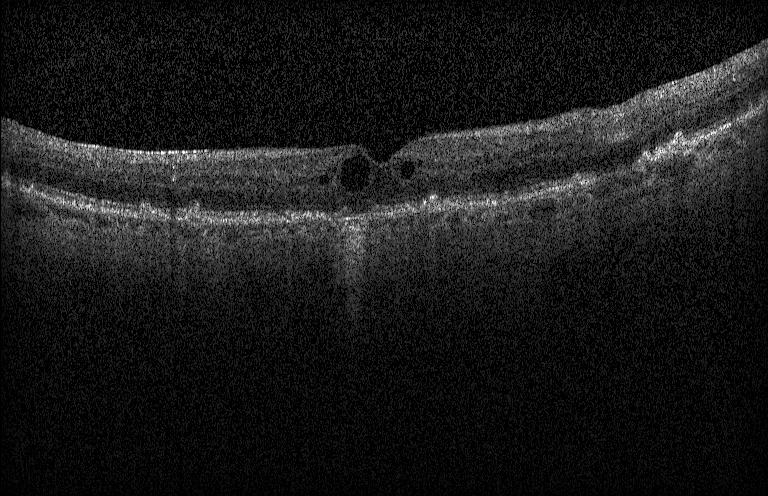 A choroidal neovascular membrane.